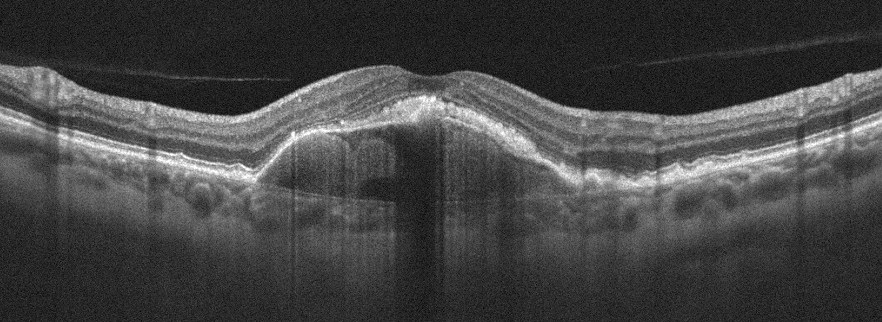

Fovea-centered, optical coherence tomography scan. OCT finding: age-related macular degeneration.